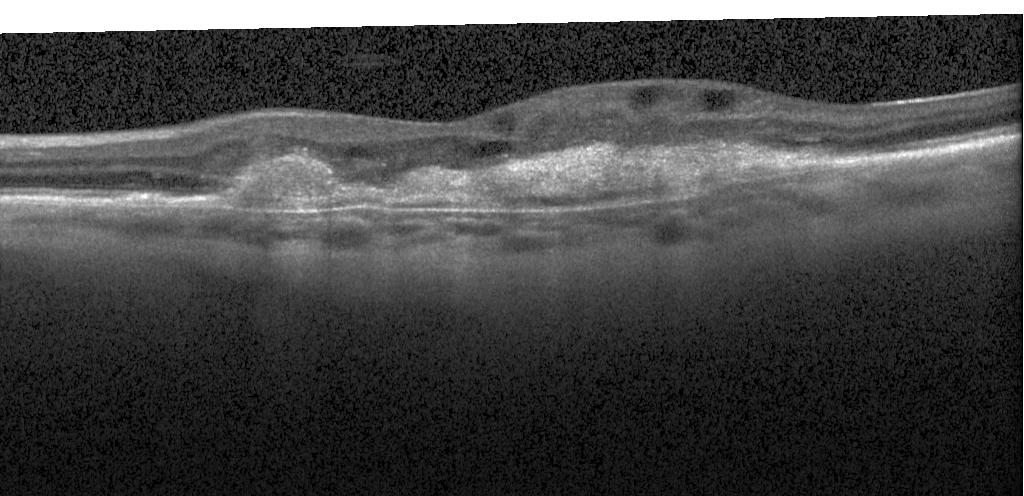
Dx: a choroidal neovascular membrane.